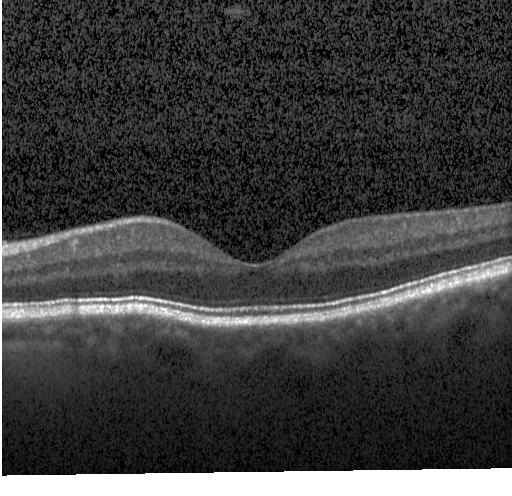
OCT B-scan — This B-scan demonstrates neither choroidal neovascularization, diabetic macular edema, nor drusen.